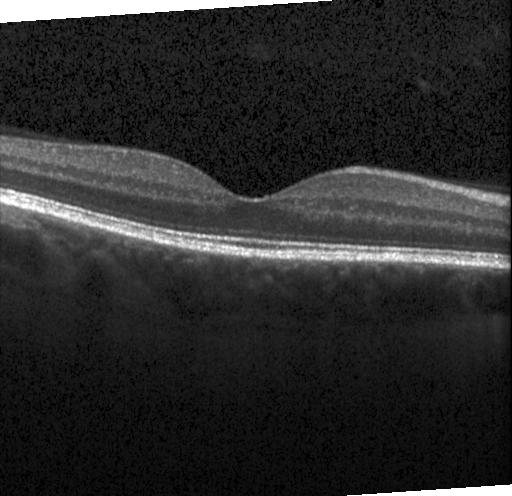 Optical coherence tomography scan. Diagnosis: no CNV, DME, or drusen.